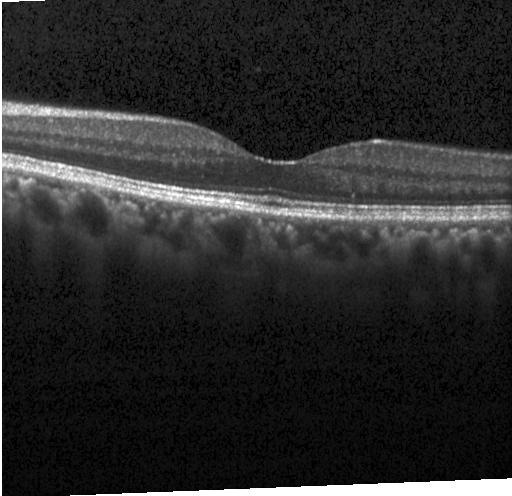
Impression: no choroidal neovascularization, no diabetic macular edema, and no drusen.